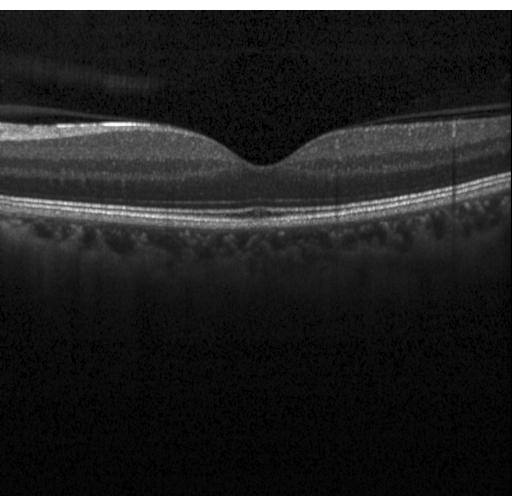
Optical coherence tomography B-scan; through the macula.
Macular OCT: neither choroidal neovascularization, diabetic macular edema, nor drusen.